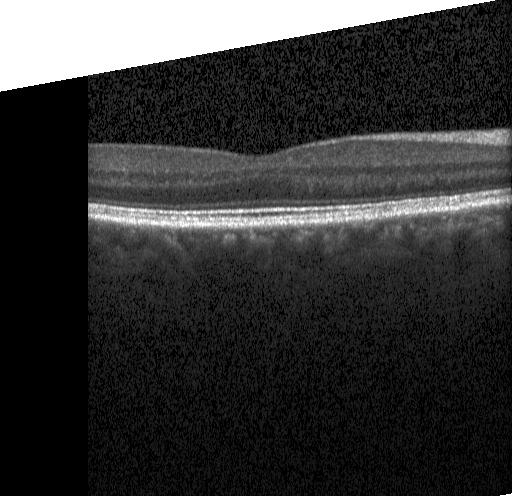

Diagnosis: no evidence of choroidal neovascularization, diabetic macular edema, or drusen.